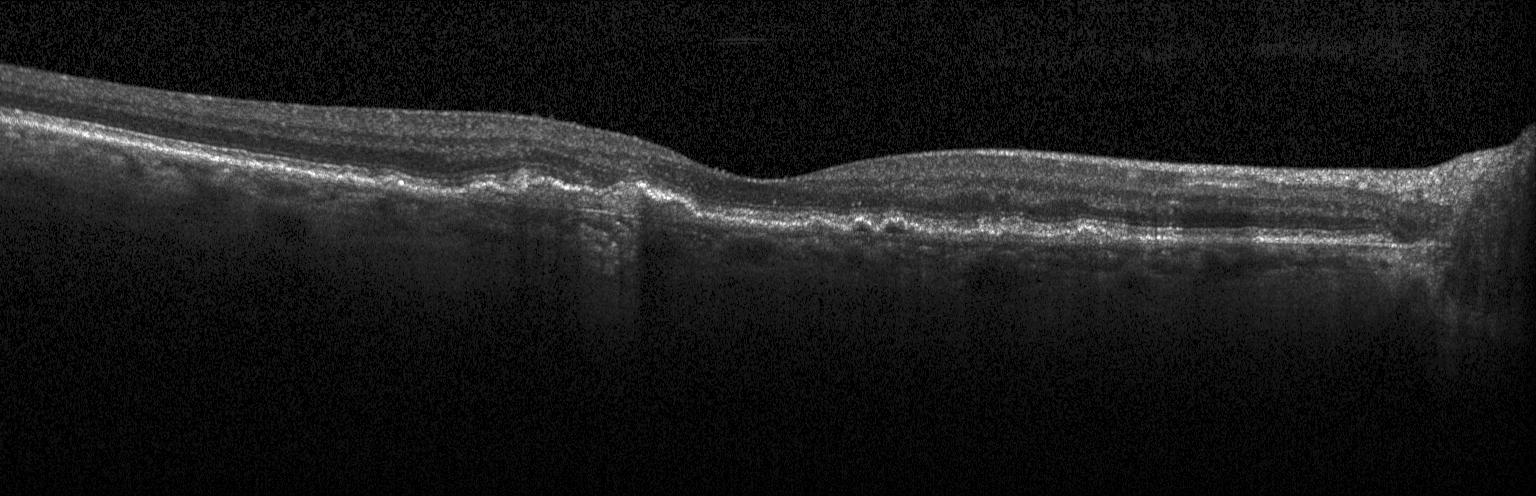
Heidelberg Spectralis · retinal OCT B-scan · spectral-domain optical coherence tomography
Finding: a choroidal neovascular membrane.